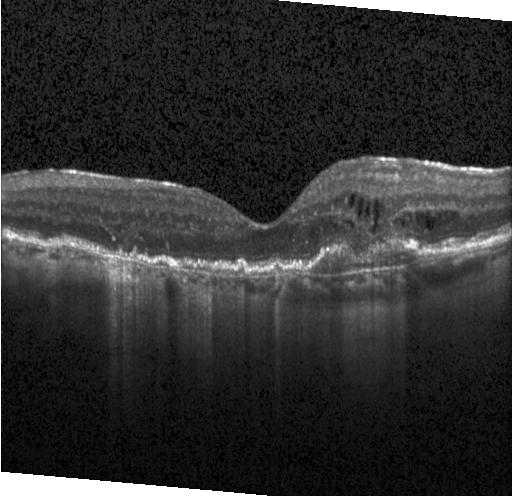
Macular OCT: CNV.